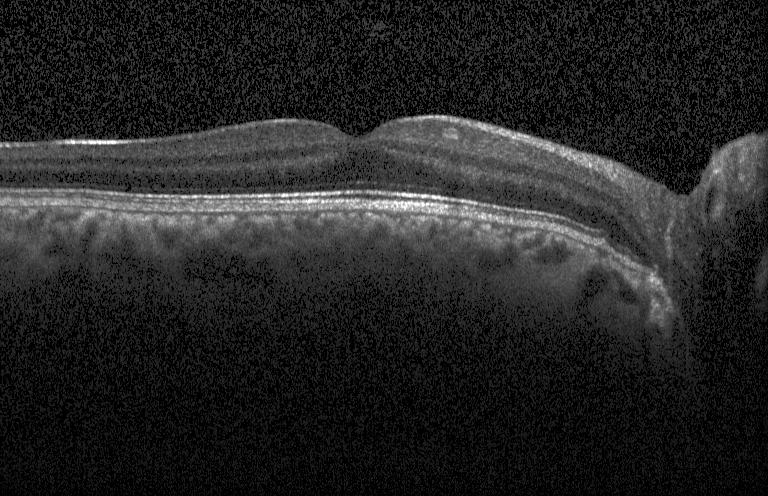 Spectral-domain optical coherence tomography; retinal OCT cross-section; centered on the fovea — This B-scan demonstrates no CNV, no DME, and no drusen.